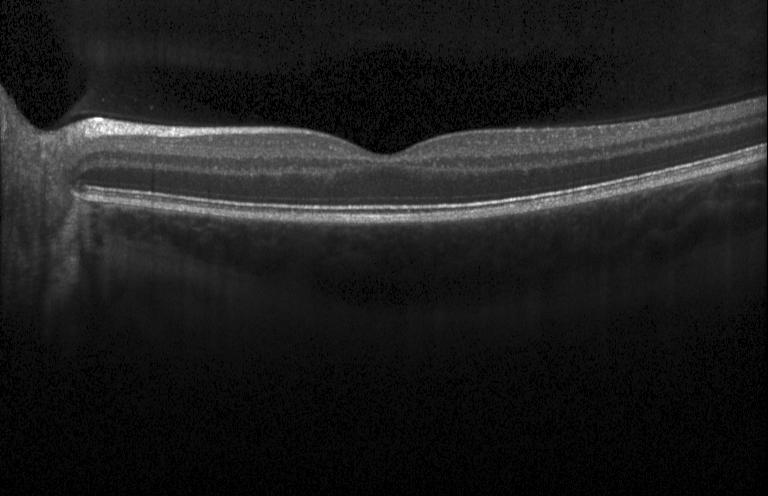
Retinal OCT B-scan. Finding: no choroidal neovascularization, diabetic macular edema, or drusen.